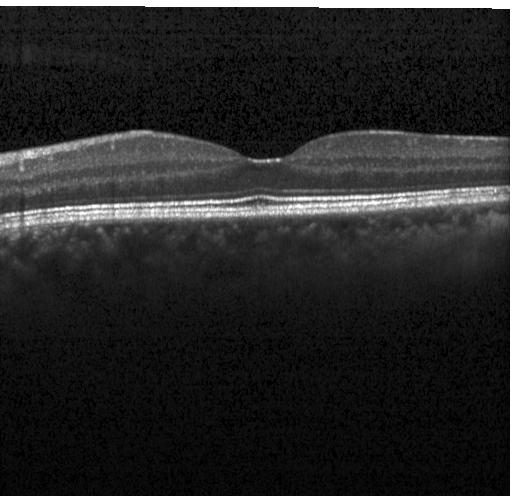 Finding: no choroidal neovascularization, diabetic macular edema, or drusen.